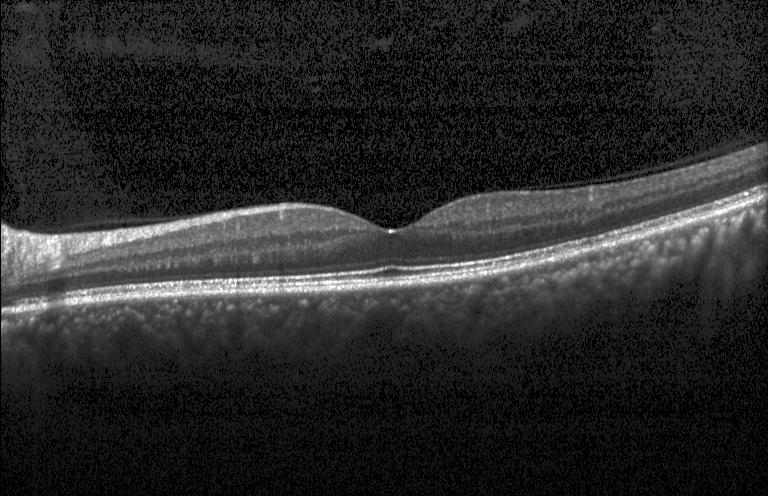
OCT scan showing no evidence of CNV, DME, or drusen.